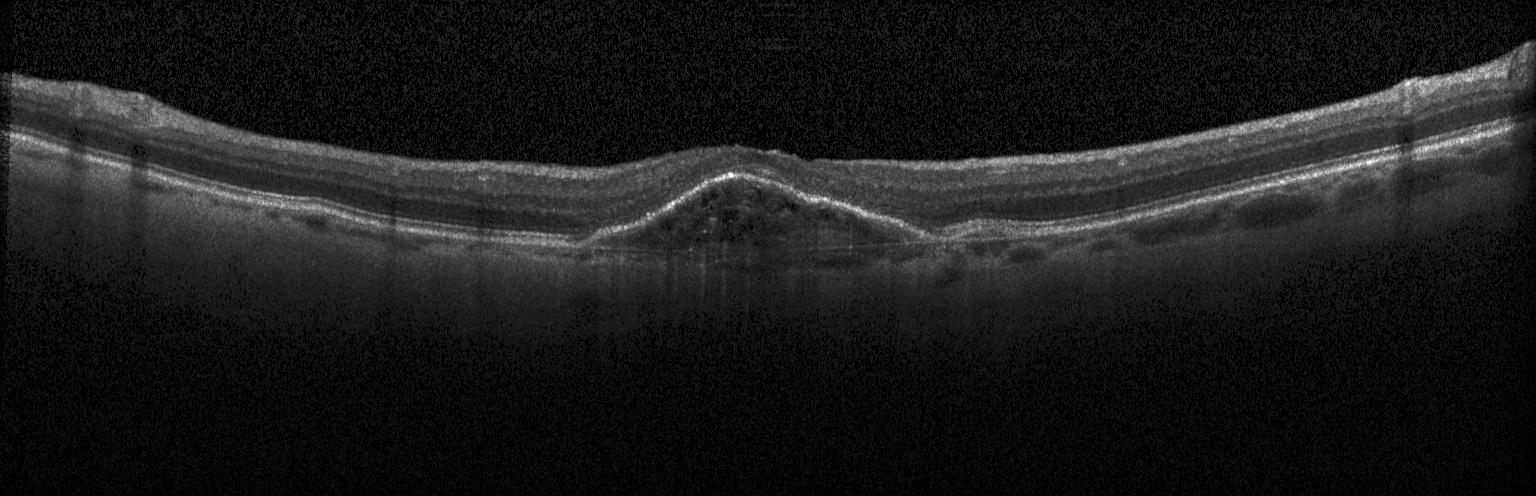

Retinal OCT B-scan. Diagnosis: choroidal neovascularization.